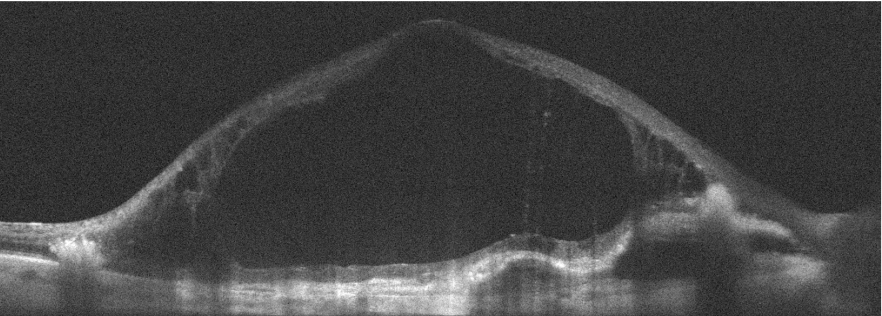

Assessment: AMD.